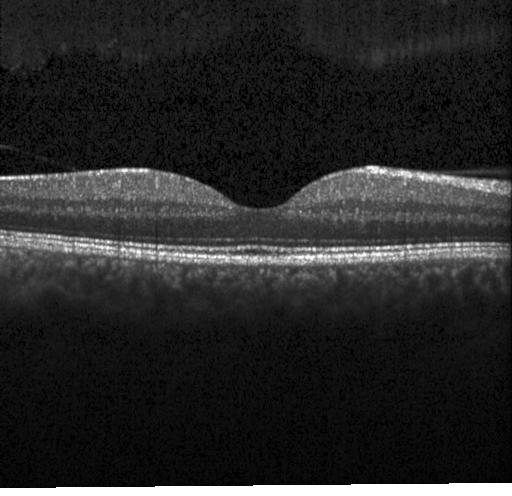 Impression: neither CNV, DME, nor drusen.